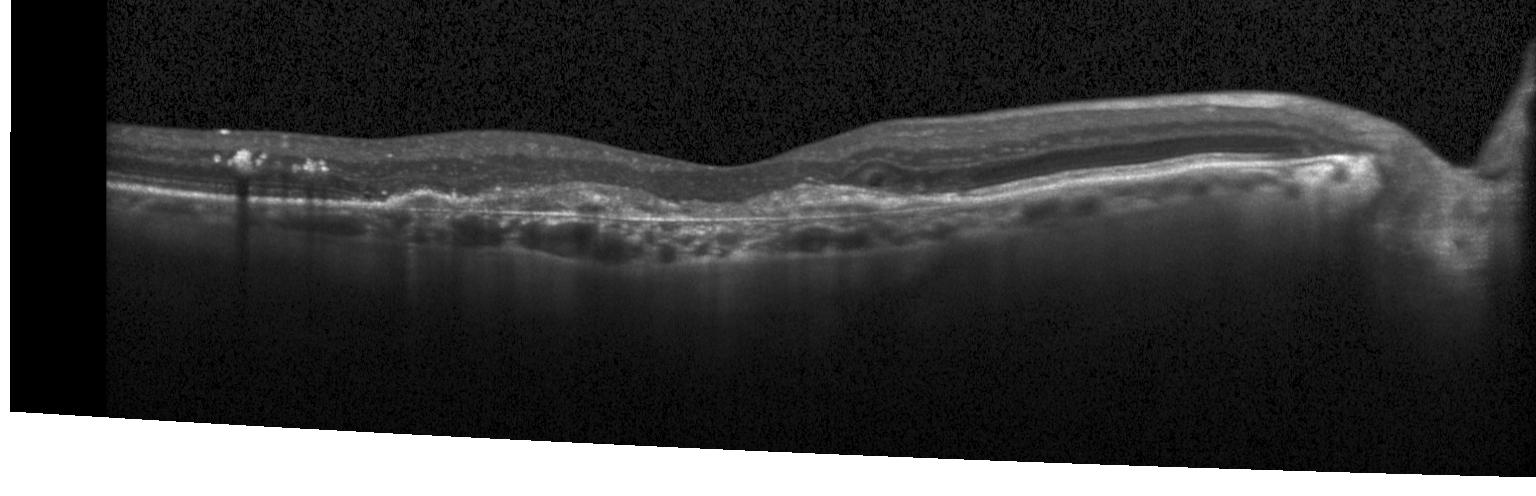 OCT B-scan; spectral-domain OCT; horizontal scan through the fovea — Impression: a choroidal neovascular membrane.